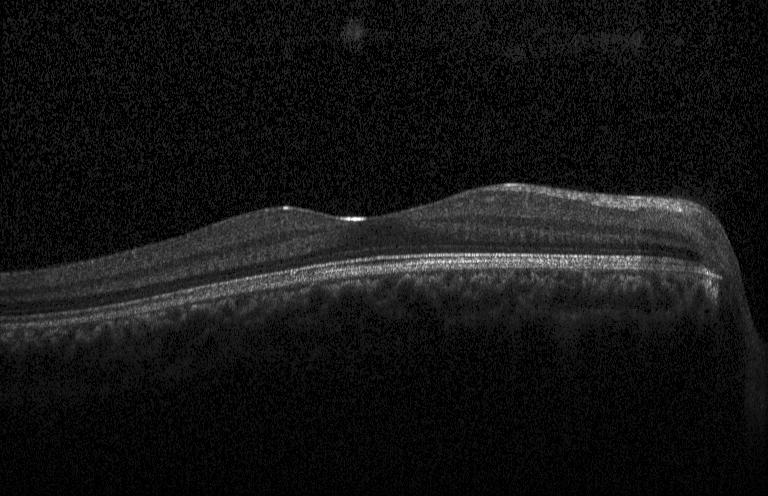
OCT B-scan, centered on the fovea. The scan shows no CNV, no DME, and no drusen.